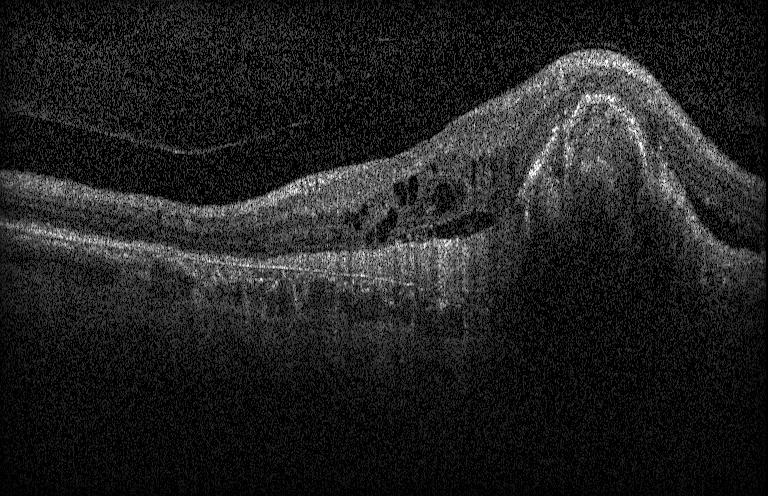 Spectral-domain optical coherence tomography; optical coherence tomography scan; centered on the fovea; Heidelberg Spectralis — Impression: a choroidal neovascular membrane.